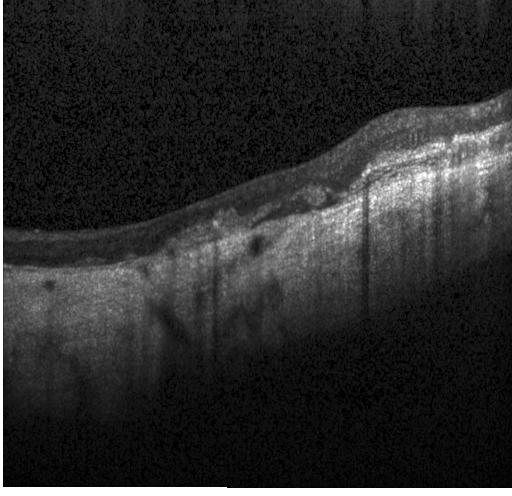
OCT line scan; Heidelberg Spectralis OCT system — Finding: a choroidal neovascular membrane.